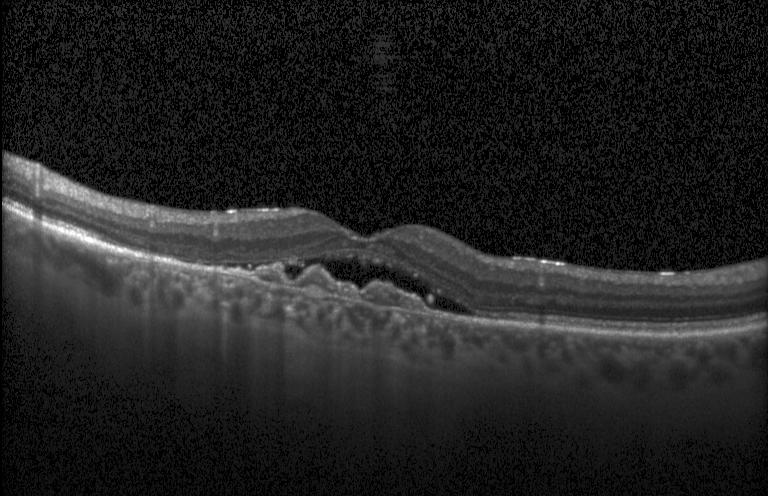

Retinal OCT B-scan.
Diagnosis: choroidal neovascularization (CNV).